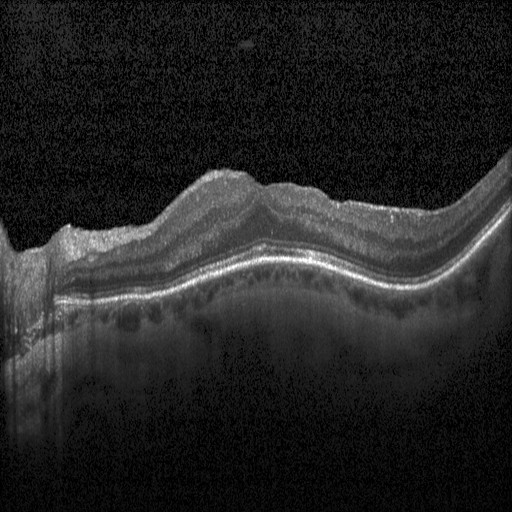

Impression: DME.